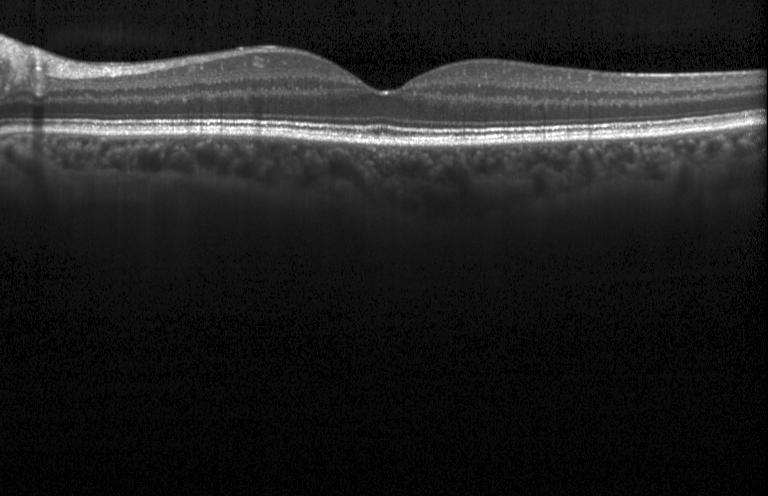 OCT line scan — Macular OCT: no choroidal neovascularization, no diabetic macular edema, and no drusen.